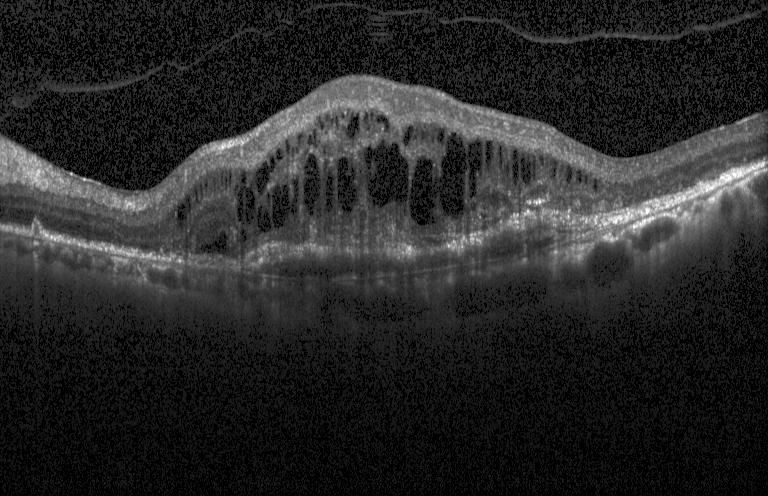 Through the macula; OCT B-scan
Finding: a choroidal neovascular membrane.